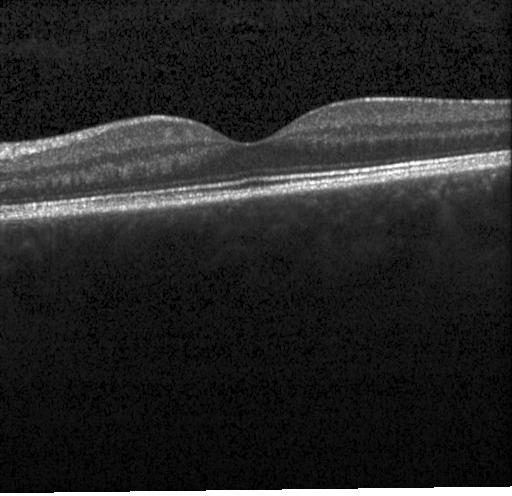 Retinal OCT B-scan · fovea-centered · spectral-domain optical coherence tomography · instrument: Heidelberg Spectralis. This B-scan demonstrates no evidence of choroidal neovascularization, diabetic macular edema, or drusen.